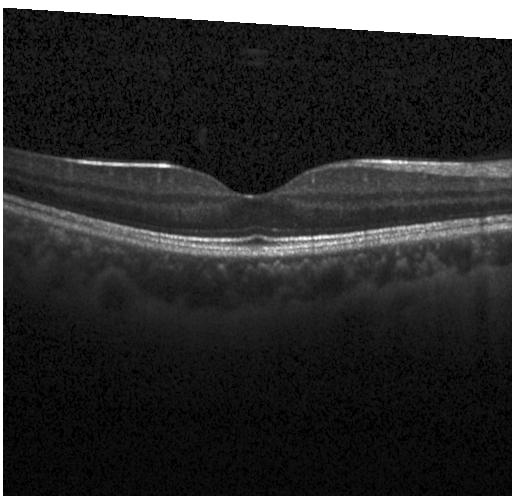 OCT B-scan. Heidelberg Spectralis. Fovea-centered. Spectral-domain optical coherence tomography. Diagnosis: no choroidal neovascularization, diabetic macular edema, or drusen.